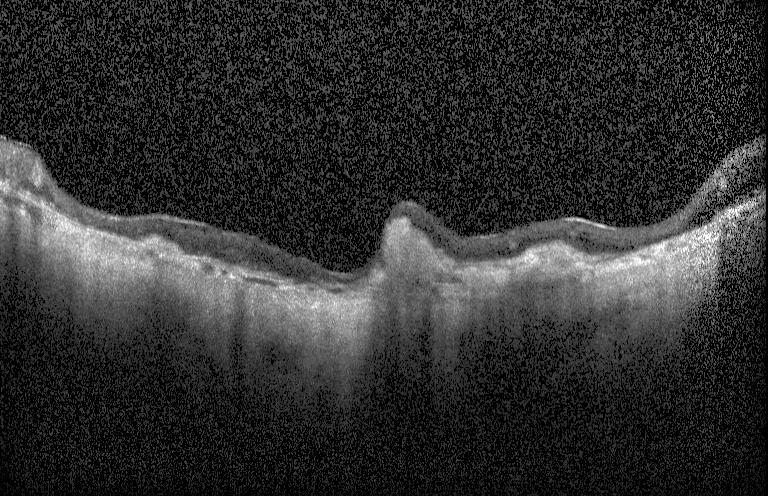

Assessment: a choroidal neovascular membrane.